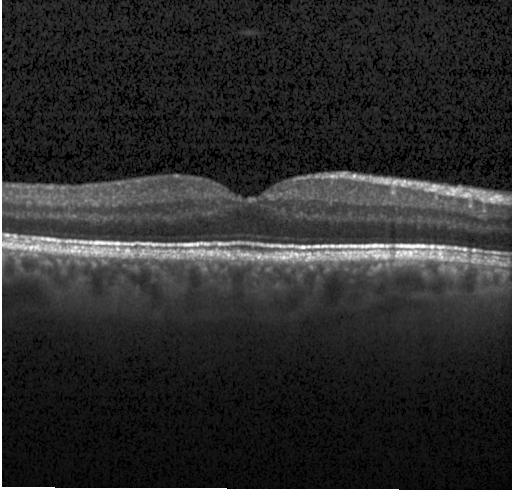

Macular scan, OCT line scan, spectral-domain optical coherence tomography — Diagnosis: no CNV, DME, or drusen.